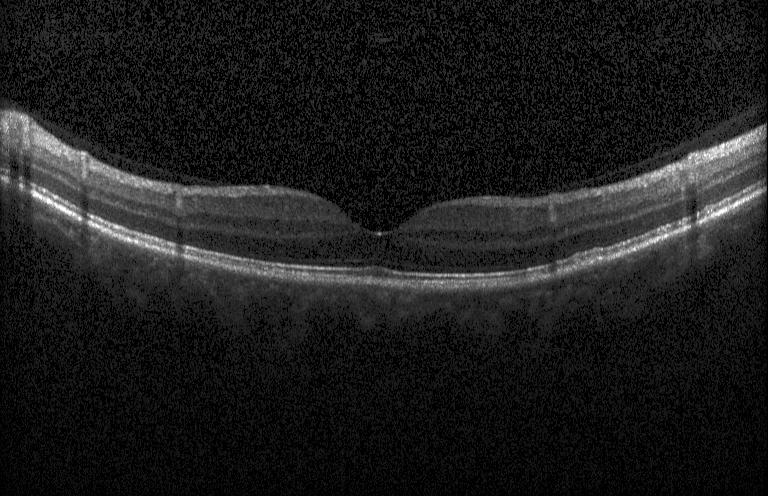
Optical coherence tomography scan. Spectral-domain optical coherence tomography. Heidelberg Spectralis — Finding: no evidence of choroidal neovascularization, diabetic macular edema, or drusen.